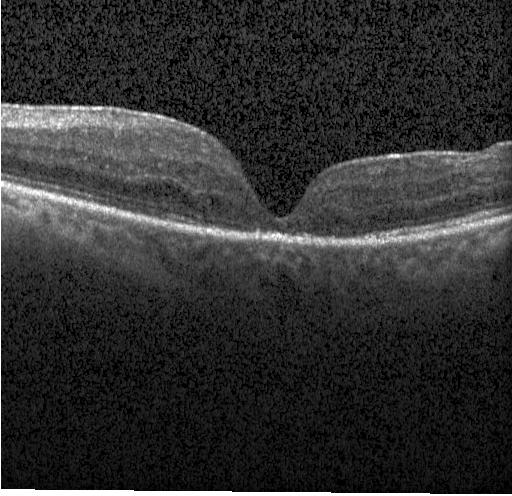

This B-scan demonstrates DME.